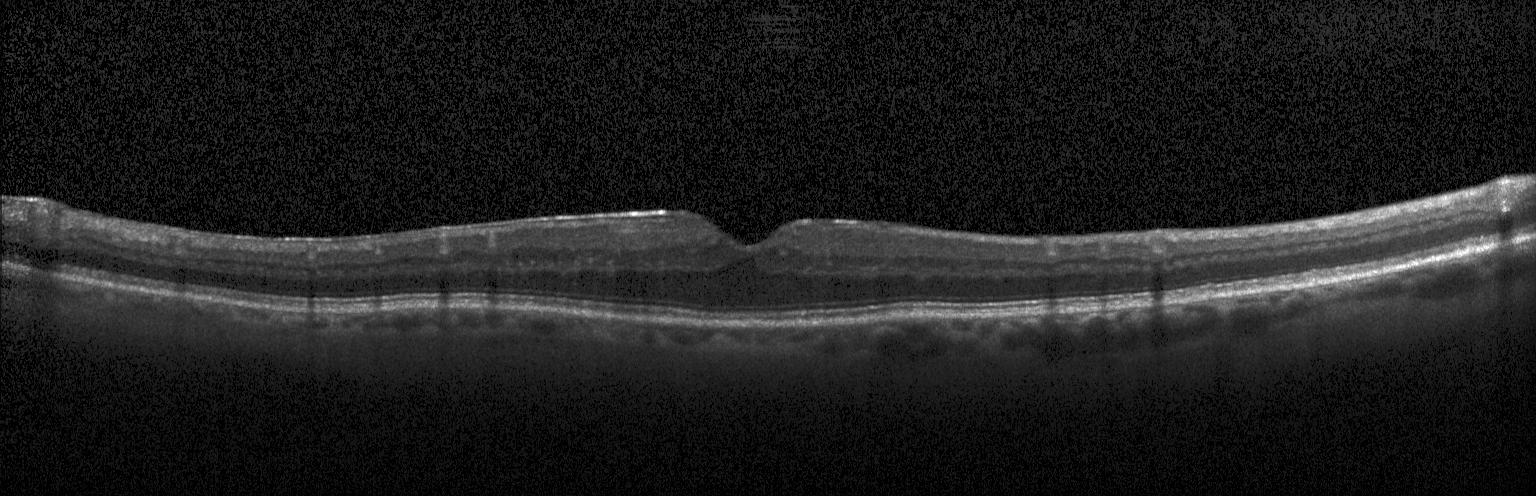
Instrument: Heidelberg Spectralis · retinal OCT B-scan · horizontal scan through the fovea · SD-OCT.
OCT finding: no choroidal neovascularization, no diabetic macular edema, and no drusen.